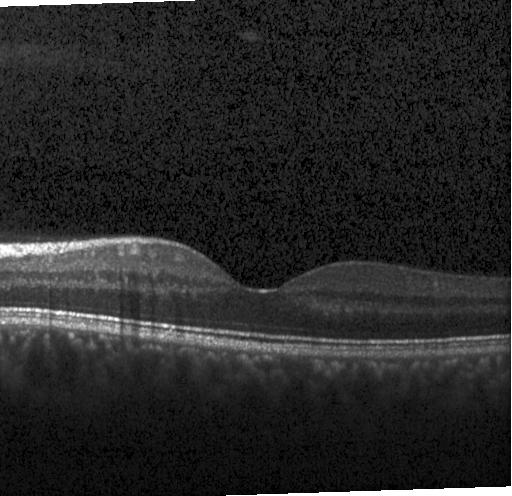 The scan shows no choroidal neovascularization, no diabetic macular edema, and no drusen.